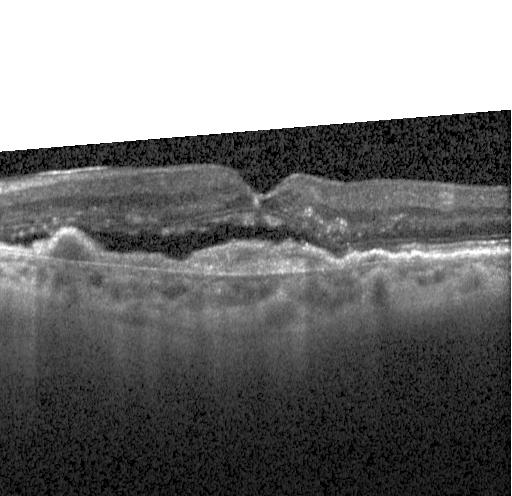

Macular OCT: a choroidal neovascular membrane.